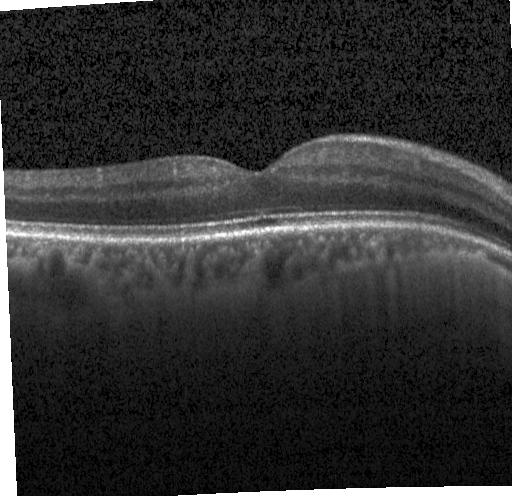
Optical coherence tomography scan. Macular scan. Heidelberg Spectralis OCT system.
Dx: no choroidal neovascularization, diabetic macular edema, or drusen.